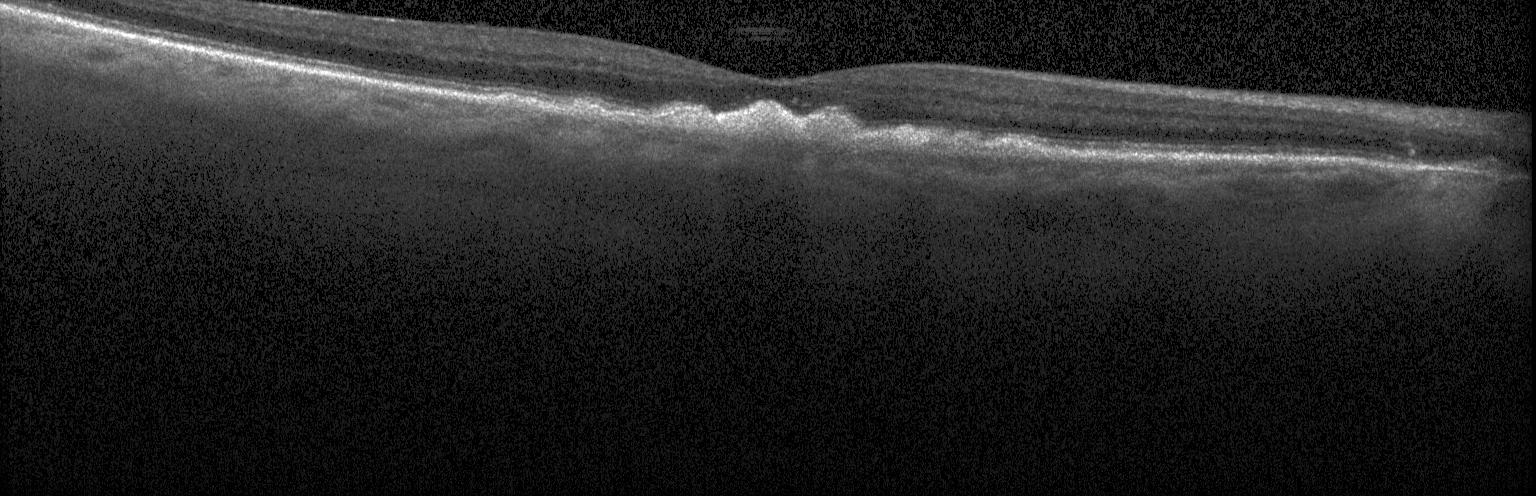
Retinal OCT B-scan. Instrument: Heidelberg Spectralis
Diagnosis: a choroidal neovascular membrane.